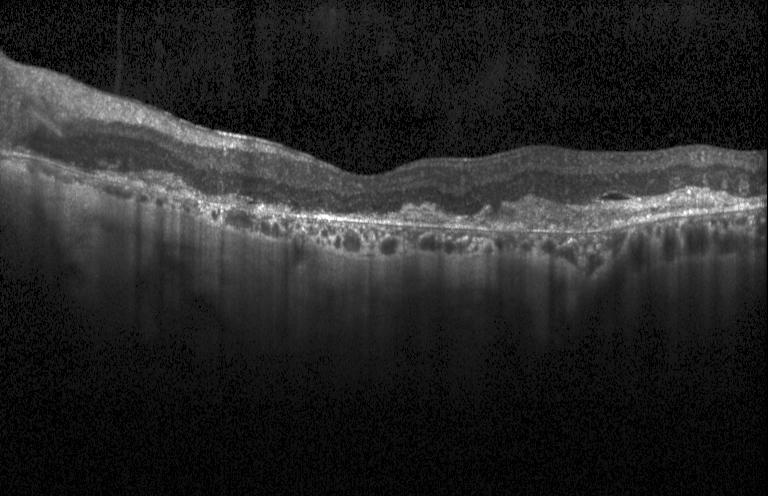
OCT line scan. Spectral-domain OCT. Instrument: Heidelberg Spectralis. Macular scan — Macular OCT: a choroidal neovascular membrane.